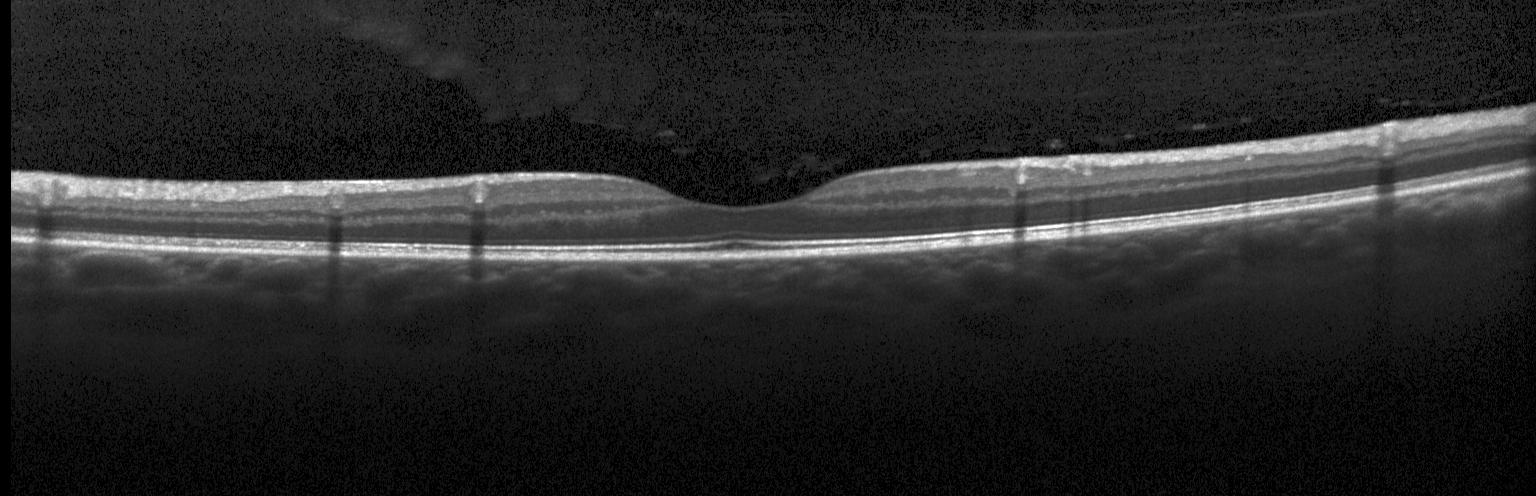
OCT B-scan. Heidelberg Spectralis OCT system. Impression: no CNV, no DME, and no drusen.